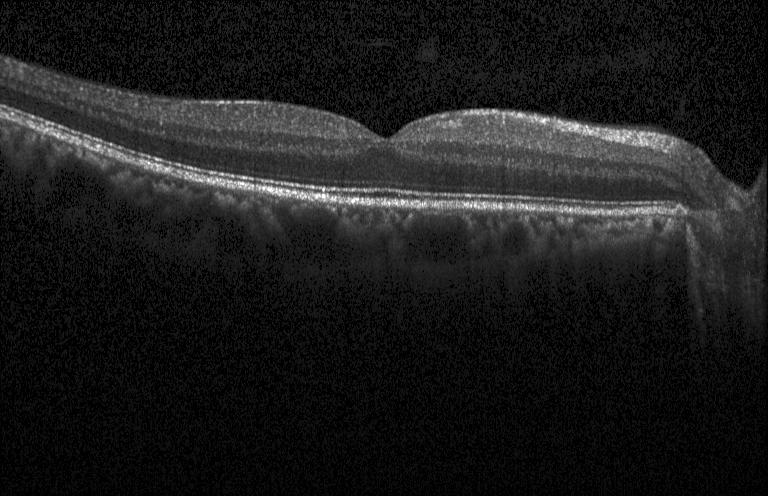 OCT B-scan showing no choroidal neovascularization, diabetic macular edema, or drusen.